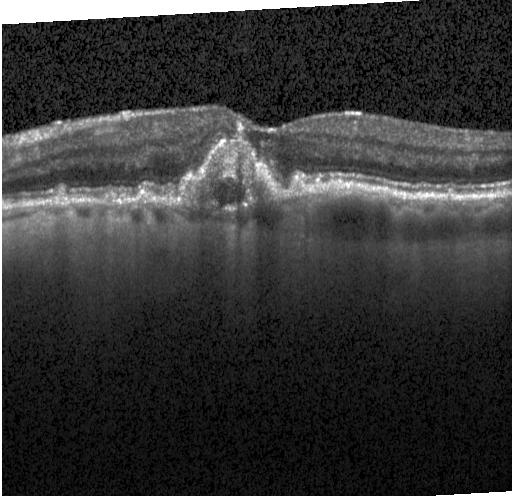 Optical coherence tomography B-scan. Heidelberg Spectralis OCT system.
Impression: CNV.